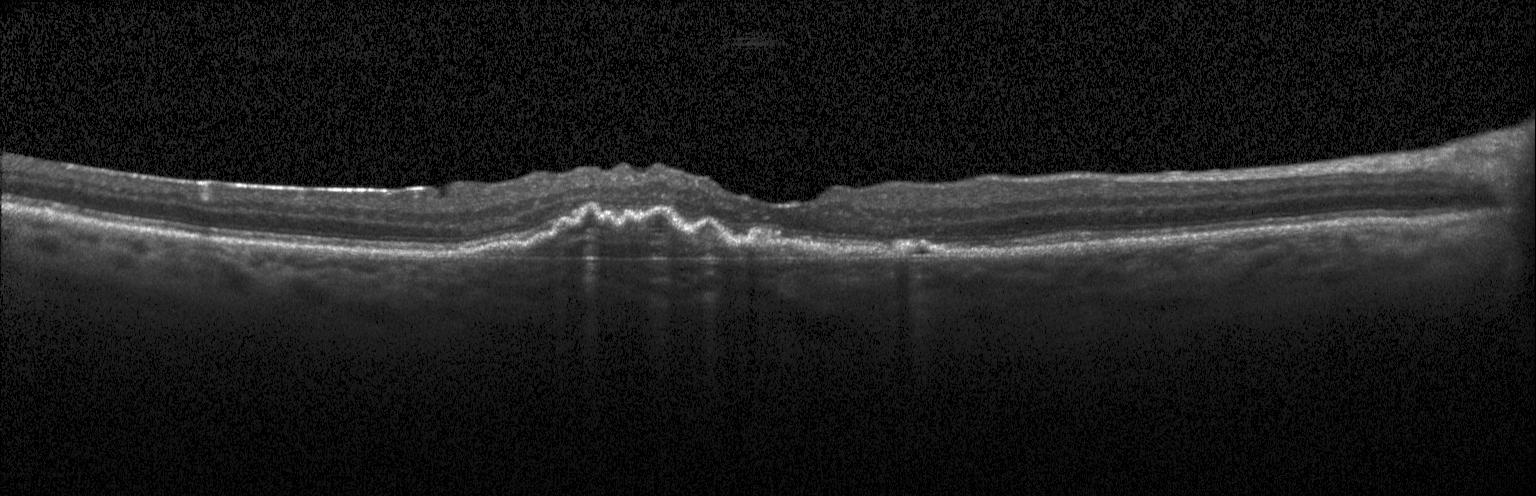

Centered on the fovea. Spectral-domain OCT. Retinal OCT B-scan. Instrument: Heidelberg Spectralis
Diagnosis: choroidal neovascularization (CNV).